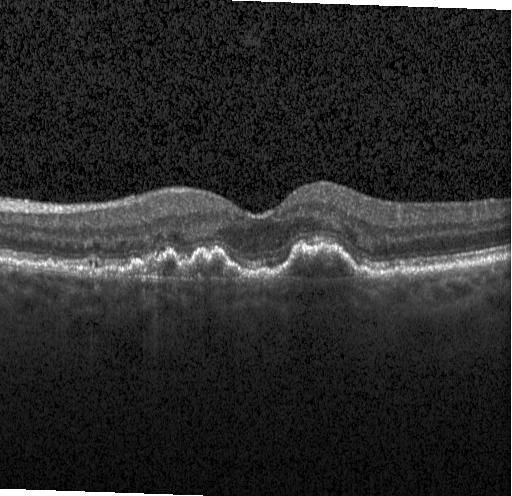

OCT B-scan; centered on the fovea
Macular OCT: a choroidal neovascular membrane.